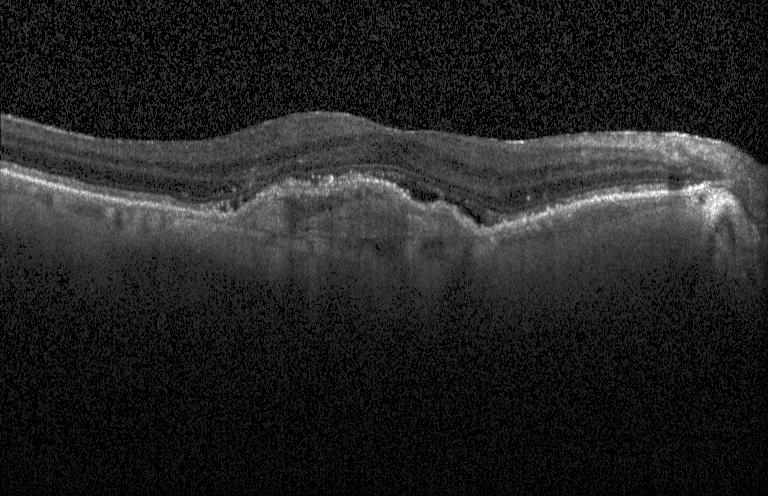
Through the macula · instrument: Heidelberg Spectralis · retinal OCT B-scan
This B-scan demonstrates a choroidal neovascular membrane.